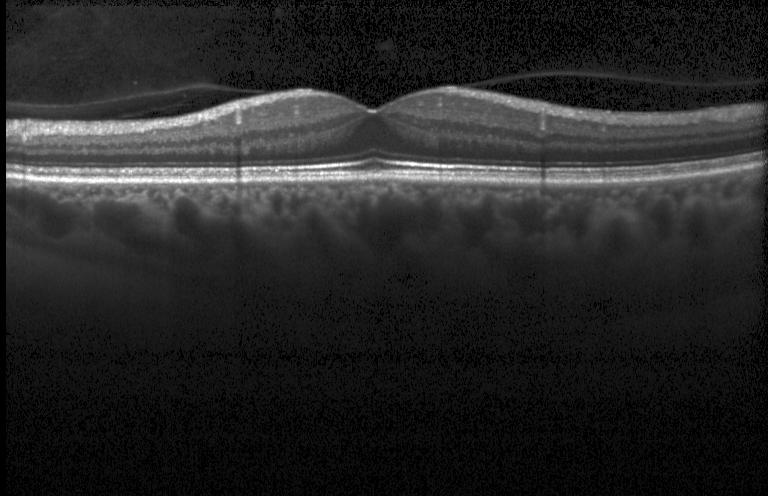 Retinal OCT B-scan, instrument: Heidelberg Spectralis — Diagnosis: no choroidal neovascularization, diabetic macular edema, or drusen.